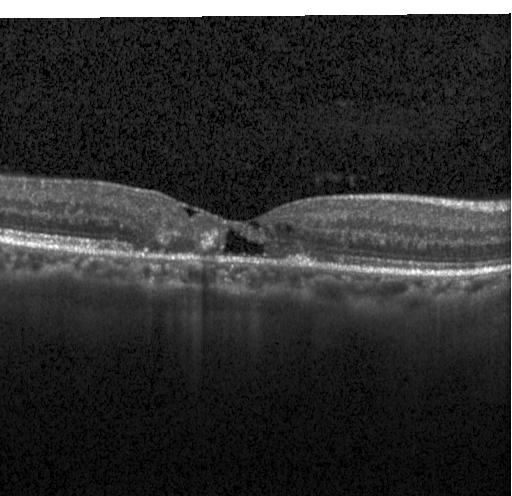 Retinal OCT B-scan
The scan shows choroidal neovascularization.